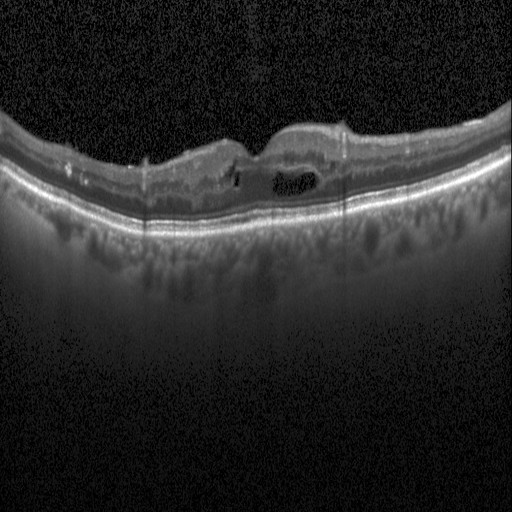 Finding: diabetic macular edema (DME).